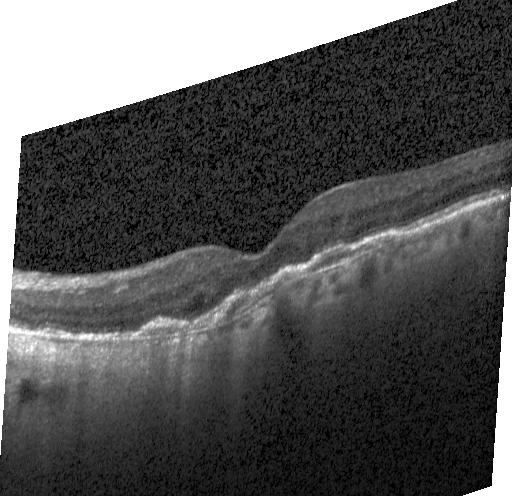
Through the macula · Heidelberg Spectralis OCT system · optical coherence tomography B-scan · spectral-domain OCT.
Diagnosis: choroidal neovascularization.